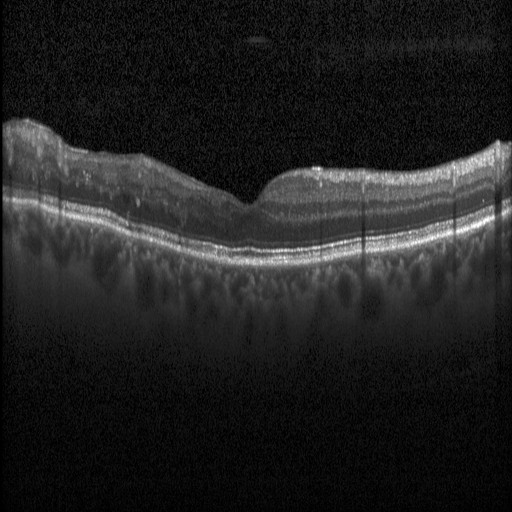 Diabetic macular edema (DME).